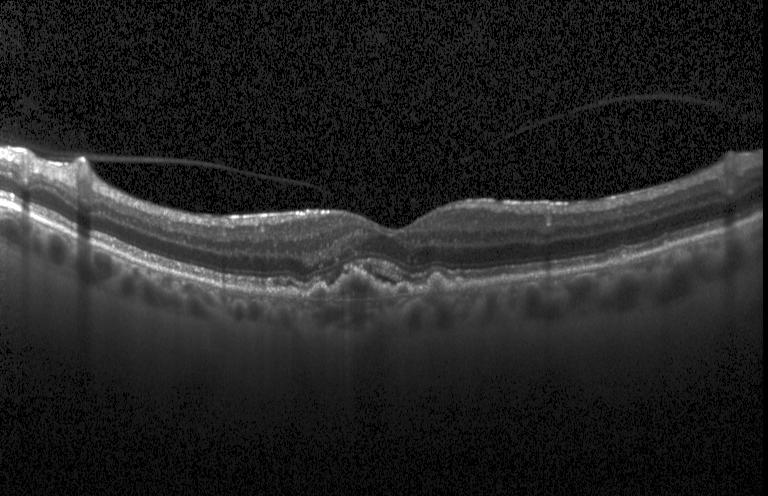

OCT scan showing choroidal neovascularization.